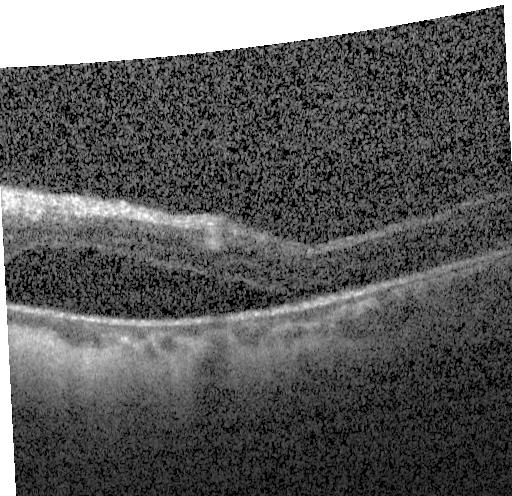 Retinal OCT cross-section showing a choroidal neovascular membrane.